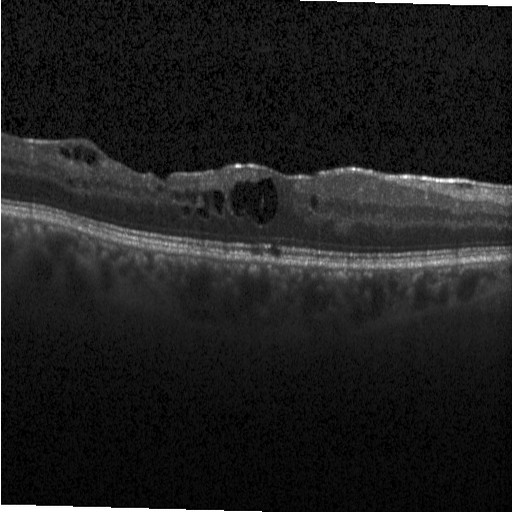

The scan shows DME.